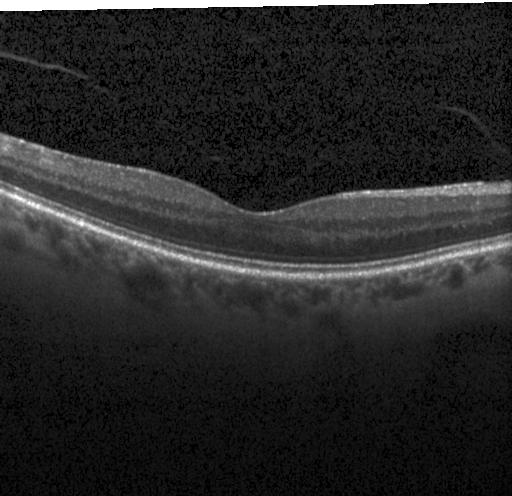 This B-scan demonstrates no choroidal neovascularization, no diabetic macular edema, and no drusen.